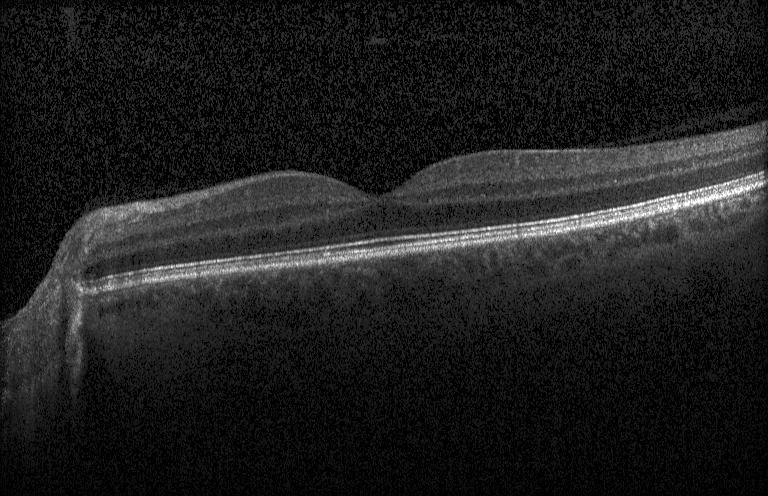
Assessment: neither choroidal neovascularization, diabetic macular edema, nor drusen.